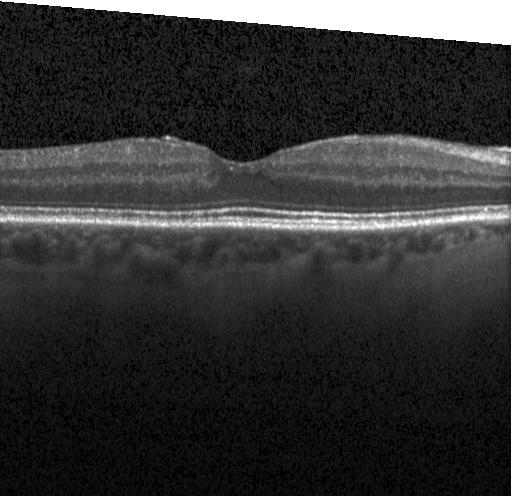
Spectral-domain OCT. OCT B-scan. Instrument: Heidelberg Spectralis. Diagnosis: no CNV, DME, or drusen.